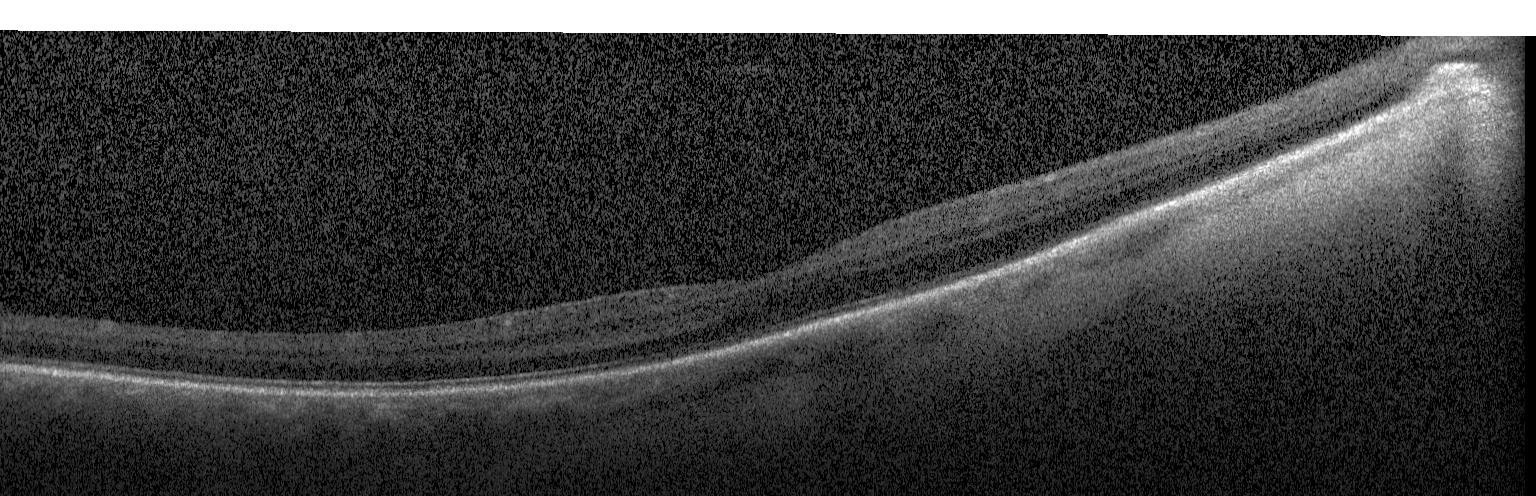 The scan shows no evidence of choroidal neovascularization, diabetic macular edema, or drusen.